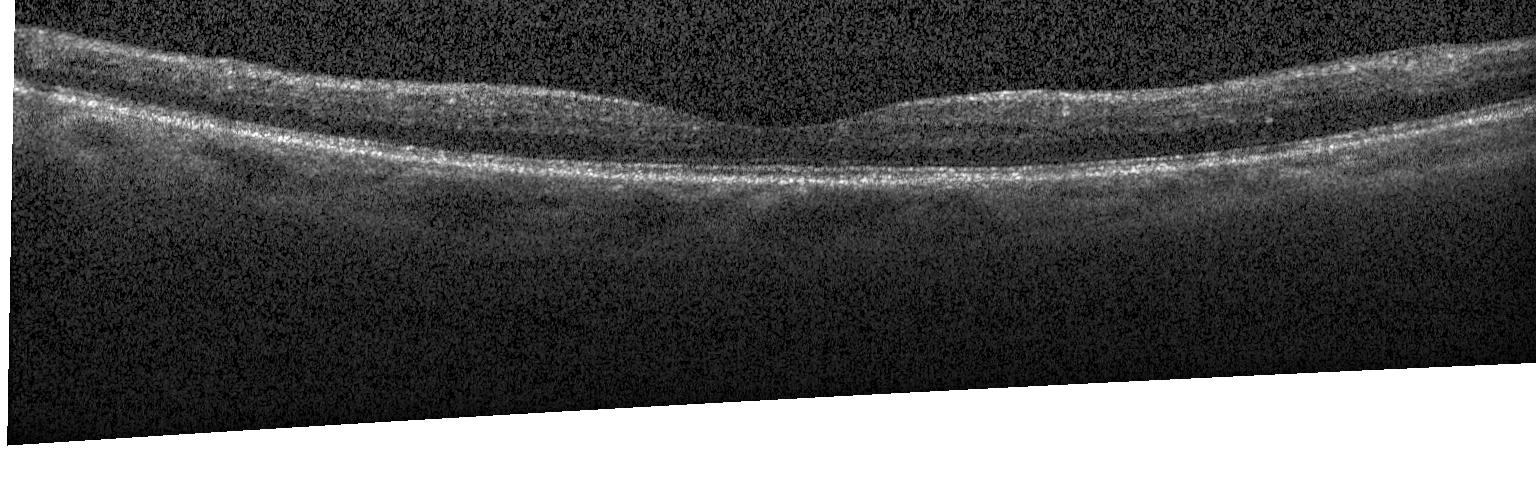 Dx: no CNV, no DME, and no drusen.